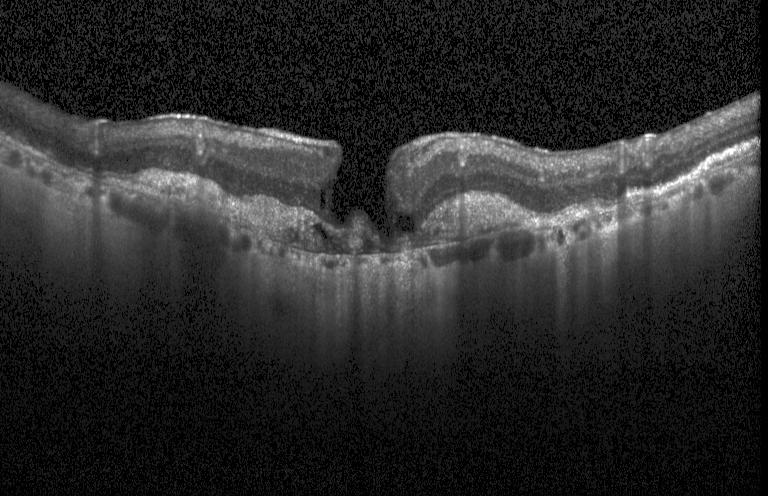

Finding: a choroidal neovascular membrane.